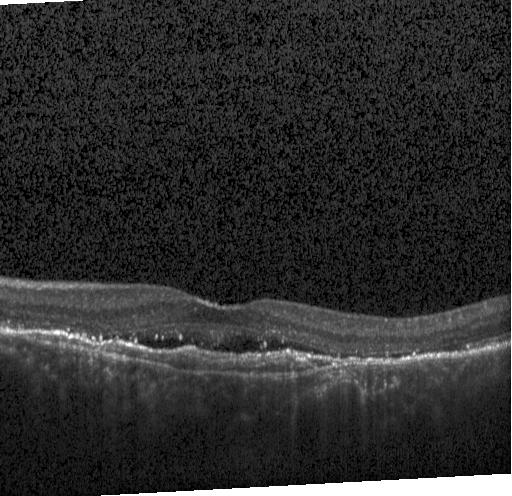

OCT B-scan. Finding: choroidal neovascularization.